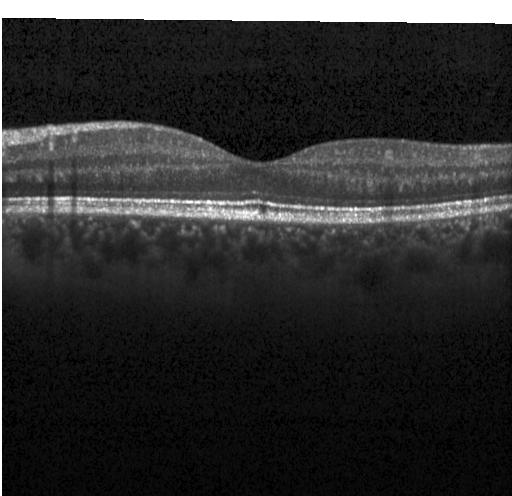

Optical coherence tomography scan; Heidelberg Spectralis OCT system; spectral-domain optical coherence tomography.
Finding: no choroidal neovascularization, no diabetic macular edema, and no drusen.